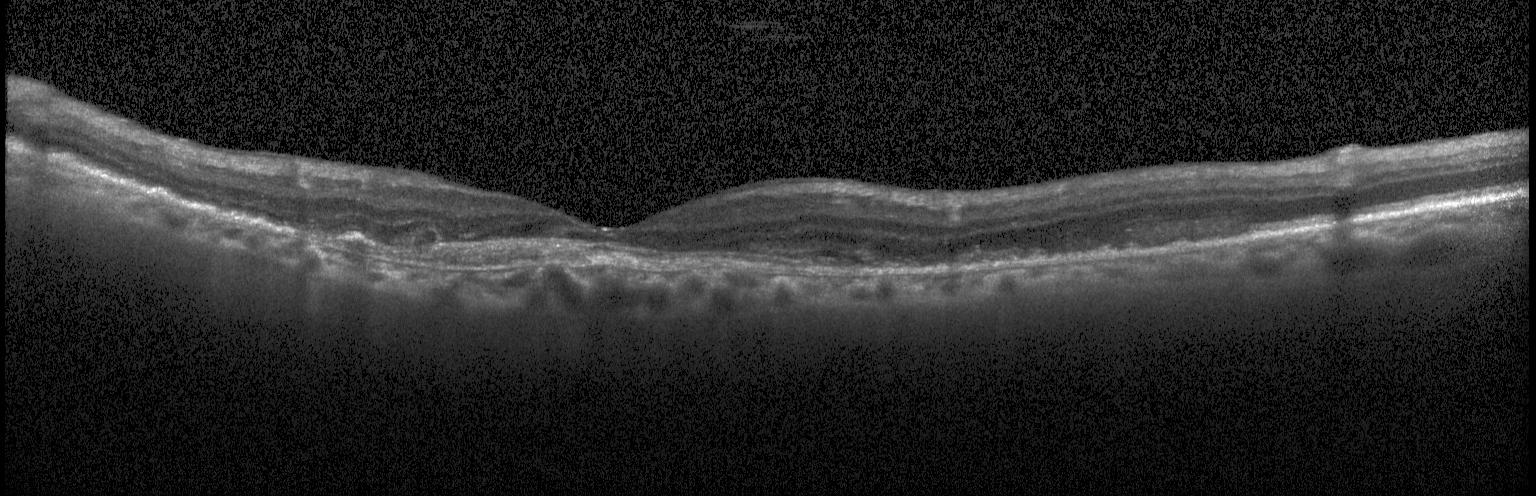 Retinal OCT B-scan; SD-OCT.
Finding: a choroidal neovascular membrane.